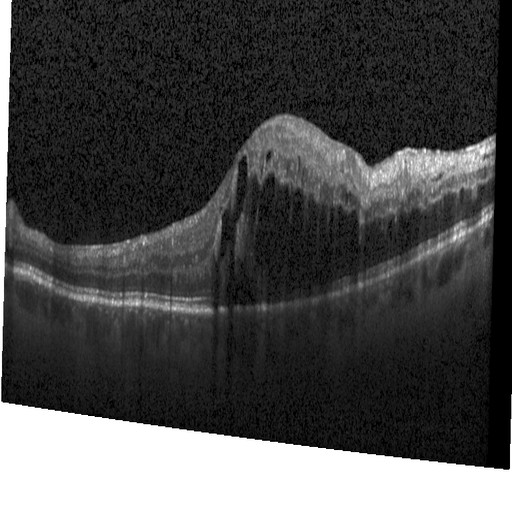
Acquired on a Heidelberg Spectralis, spectral-domain OCT, horizontal scan through the fovea, OCT line scan — The scan shows DME.